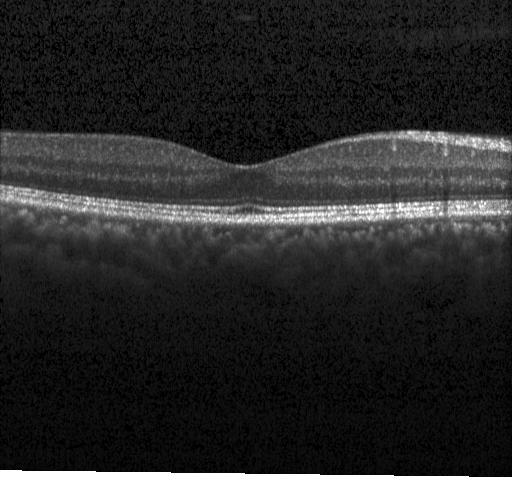
Optical coherence tomography scan · Heidelberg Spectralis OCT system · spectral-domain OCT · centered on the fovea. Finding: neither CNV, DME, nor drusen.